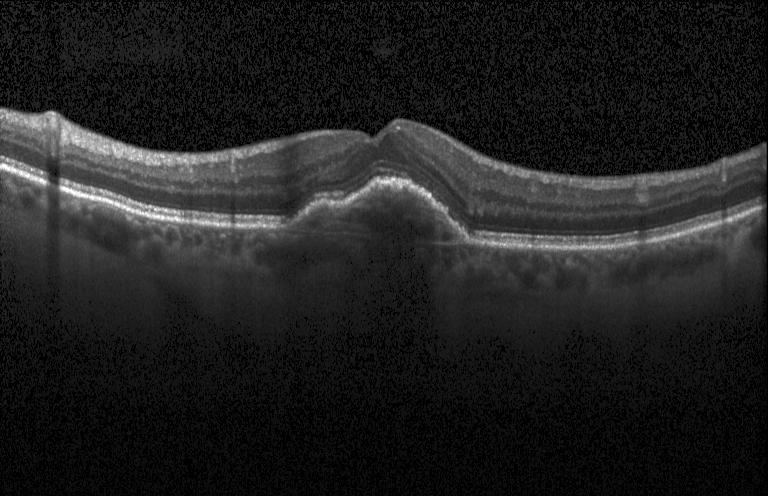
Impression: a choroidal neovascular membrane.